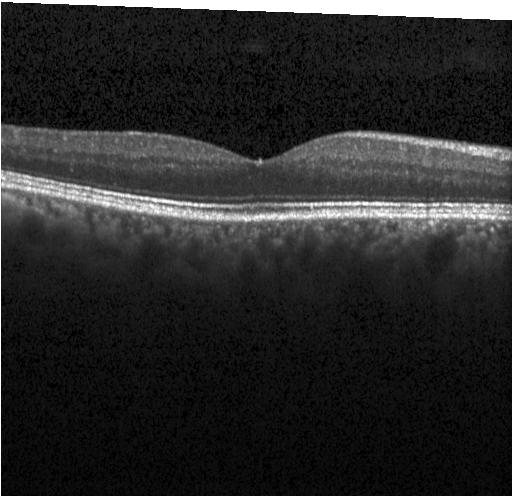
Retinal OCT cross-section, SD-OCT, through the macula, Heidelberg Spectralis OCT system.
This B-scan demonstrates no choroidal neovascularization, no diabetic macular edema, and no drusen.